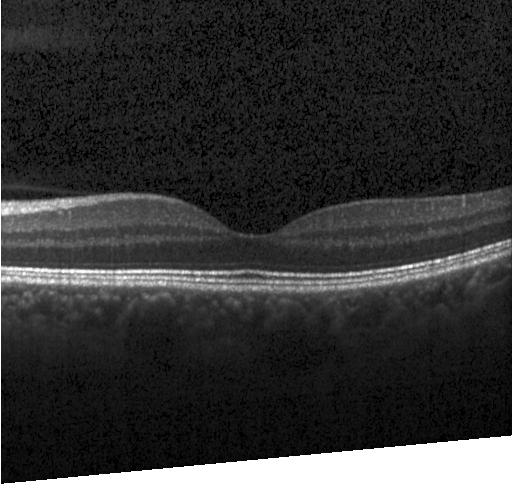 Heidelberg Spectralis OCT system; macular scan; OCT B-scan
Diagnosis: no evidence of CNV, DME, or drusen.